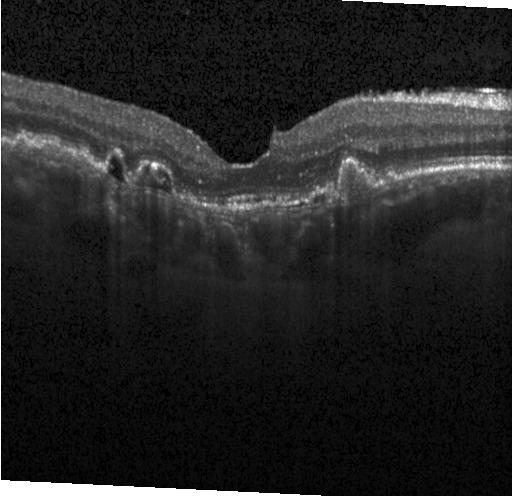 Retinal OCT B-scan — Diagnosis: a choroidal neovascular membrane.